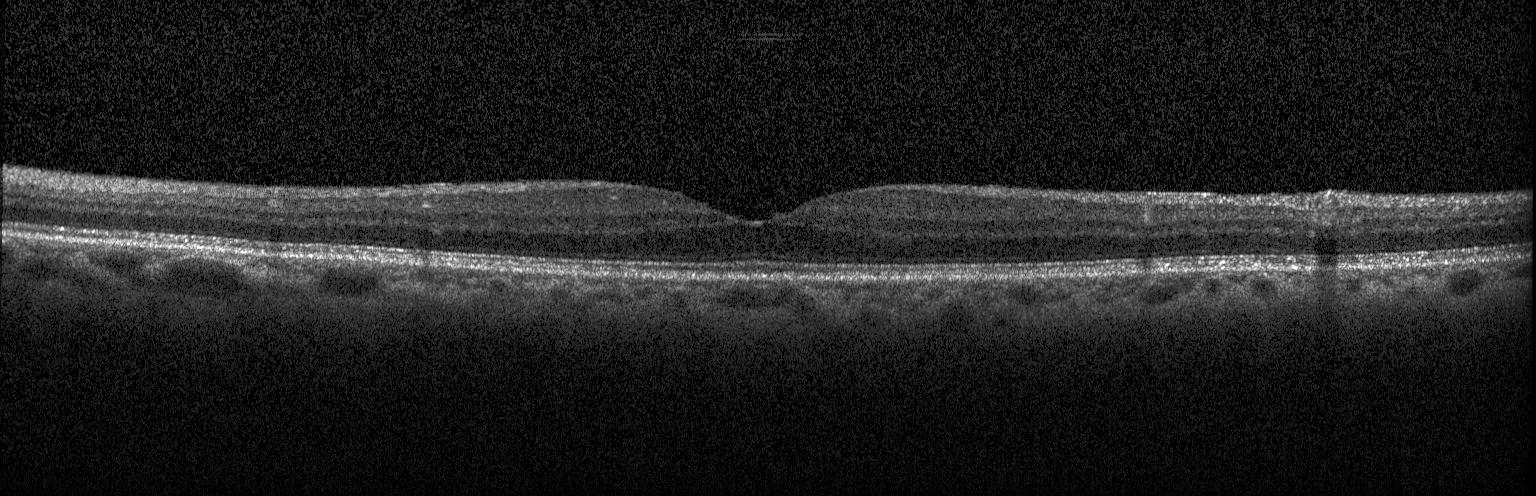

Impression: no choroidal neovascularization, no diabetic macular edema, and no drusen.